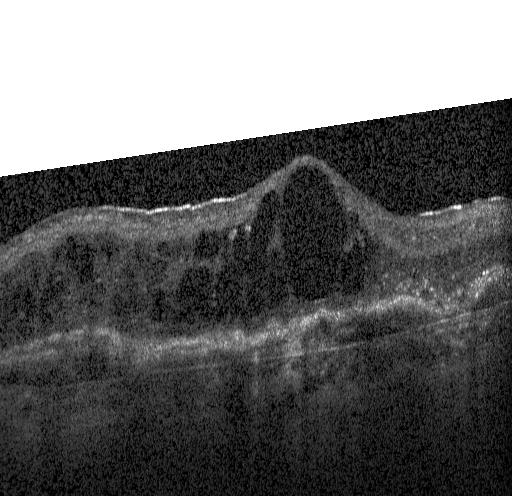 Macular OCT: a choroidal neovascular membrane.